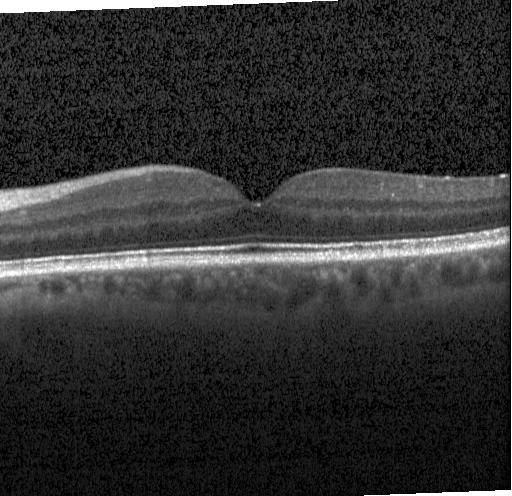

OCT line scan. Finding: no choroidal neovascularization, no diabetic macular edema, and no drusen.